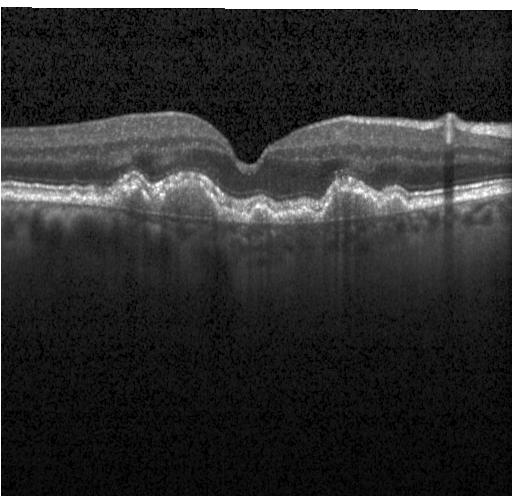
Horizontal scan through the fovea, acquired on a Heidelberg Spectralis, optical coherence tomography scan
Finding: drusen.